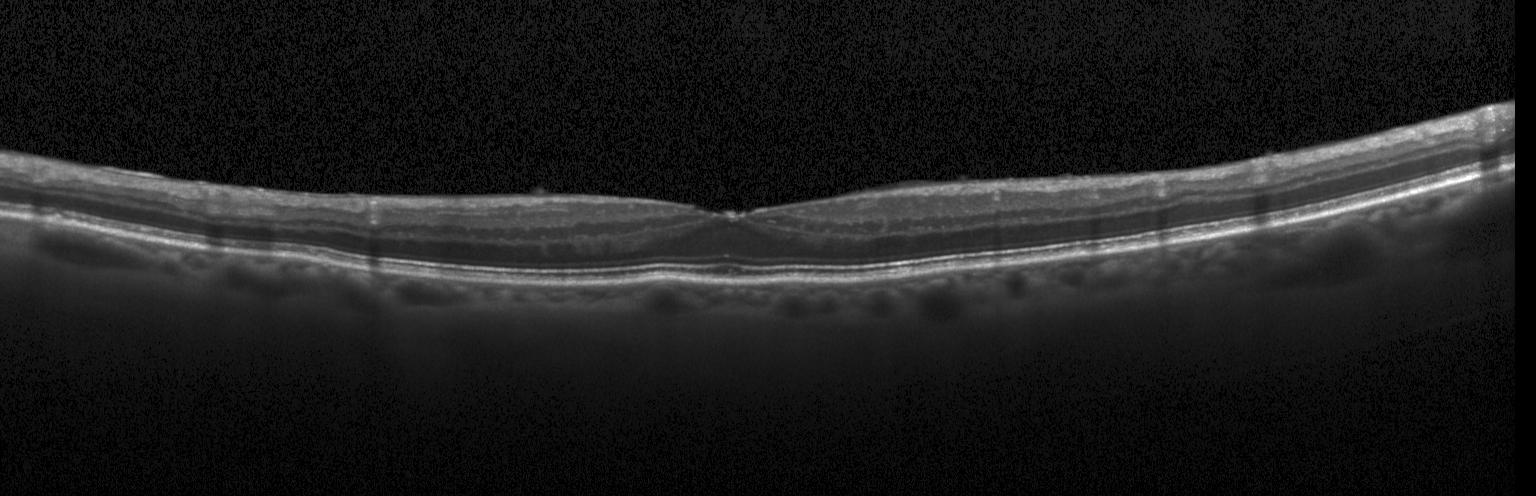
Impression: no evidence of choroidal neovascularization, diabetic macular edema, or drusen.